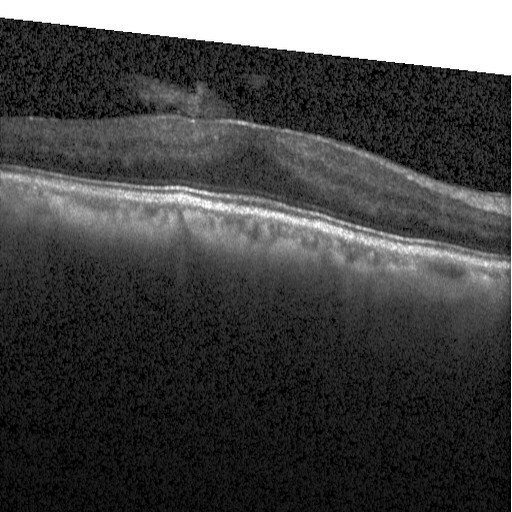 Diagnosis: DME.